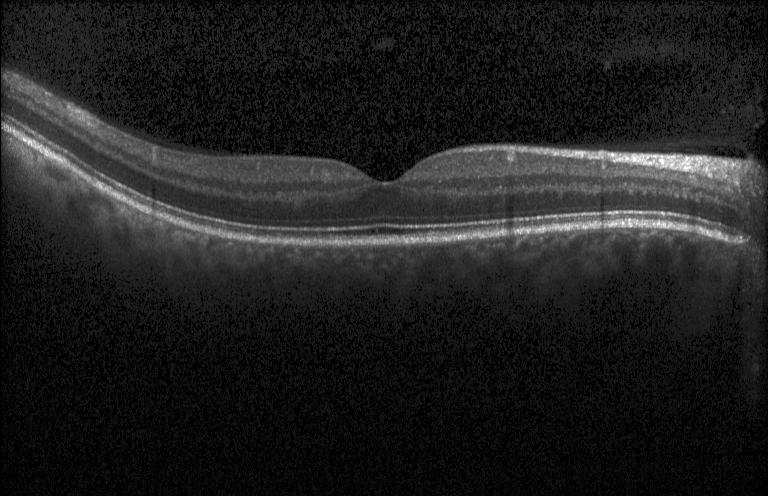 OCT scan showing neither choroidal neovascularization, diabetic macular edema, nor drusen.